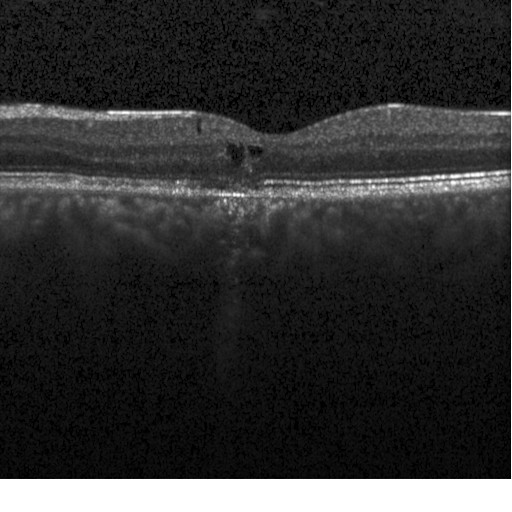
Heidelberg Spectralis · optical coherence tomography B-scan · fovea-centered
Finding: diabetic macular edema (DME).